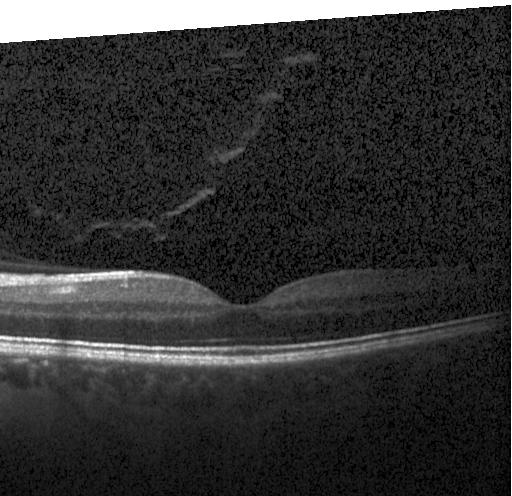

OCT line scan.
Impression: no evidence of choroidal neovascularization, diabetic macular edema, or drusen.